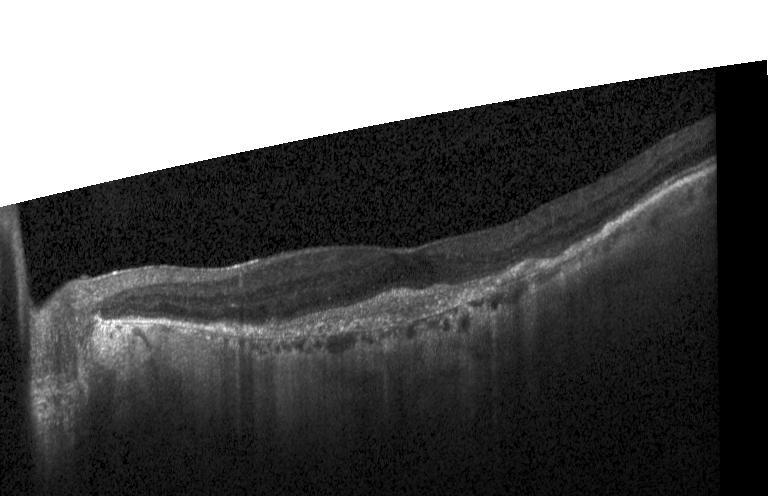

Instrument: Heidelberg Spectralis, centered on the fovea, optical coherence tomography scan — Finding: choroidal neovascularization (CNV).